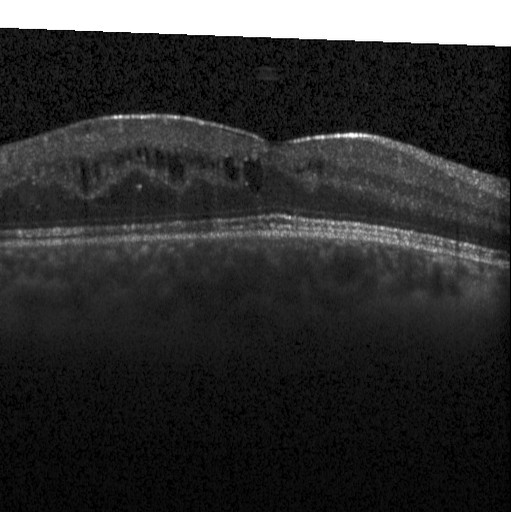

Horizontal scan through the fovea. Retinal OCT cross-section. Acquired on a Heidelberg Spectralis — Finding: diabetic macular edema (DME).